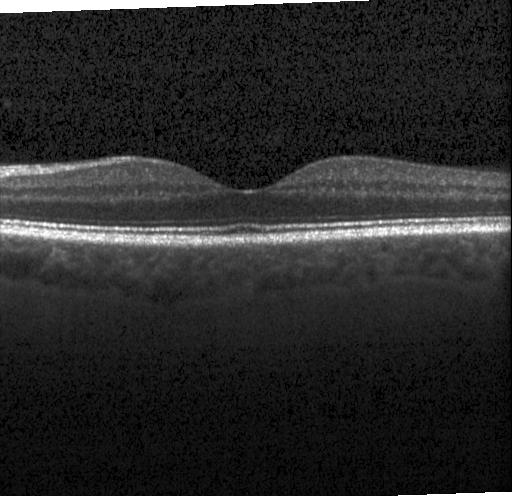 Spectral-domain OCT B-scan: no CNV, DME, or drusen.